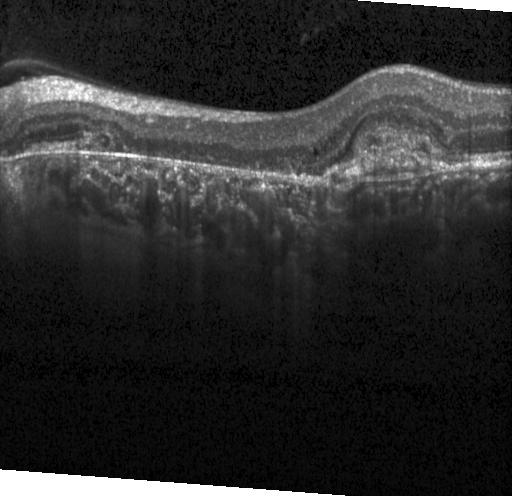 Finding: choroidal neovascularization (CNV).